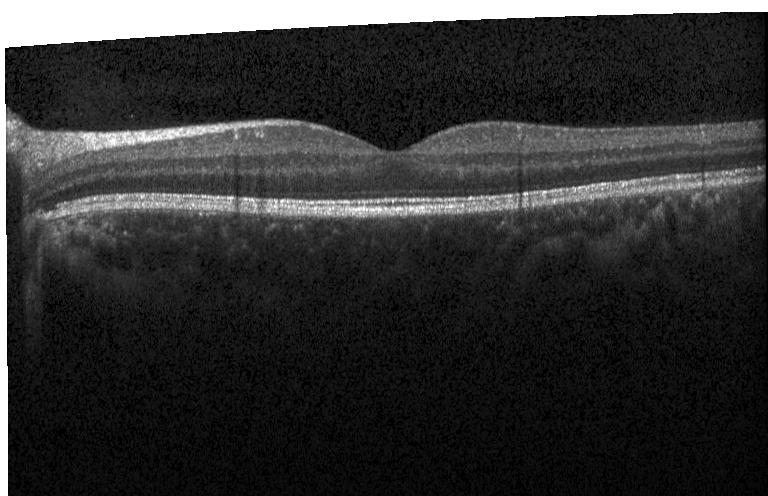
Optical coherence tomography scan; SD-OCT; horizontal scan through the fovea — Finding: no choroidal neovascularization, no diabetic macular edema, and no drusen.